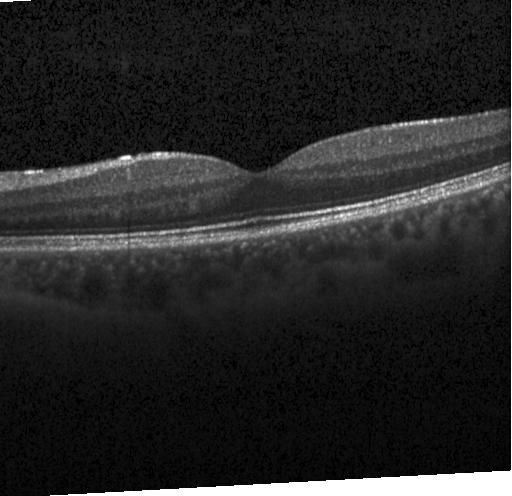 Heidelberg Spectralis OCT system; OCT line scan; macular scan
Diagnosis: neither choroidal neovascularization, diabetic macular edema, nor drusen.